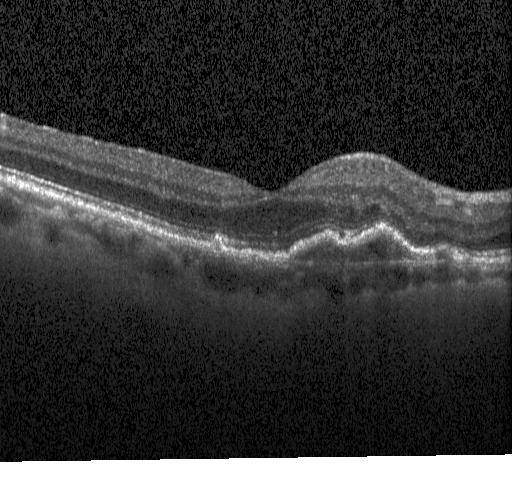 Fovea-centered · optical coherence tomography scan · spectral-domain OCT · Heidelberg Spectralis
Impression: CNV.